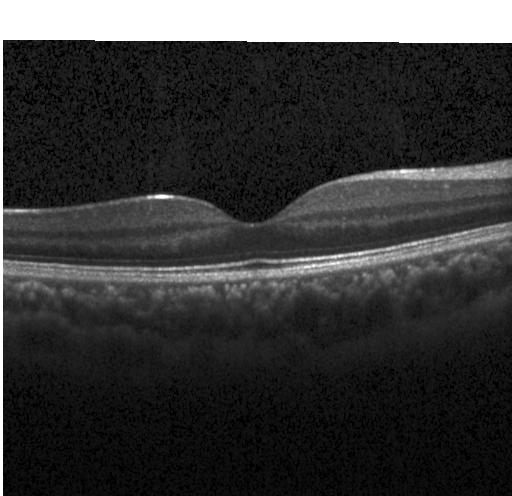

Diagnosis: no choroidal neovascularization, no diabetic macular edema, and no drusen.